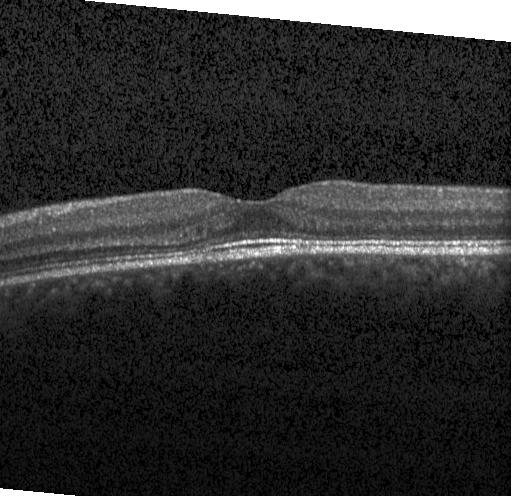 The scan shows no choroidal neovascularization, diabetic macular edema, or drusen.